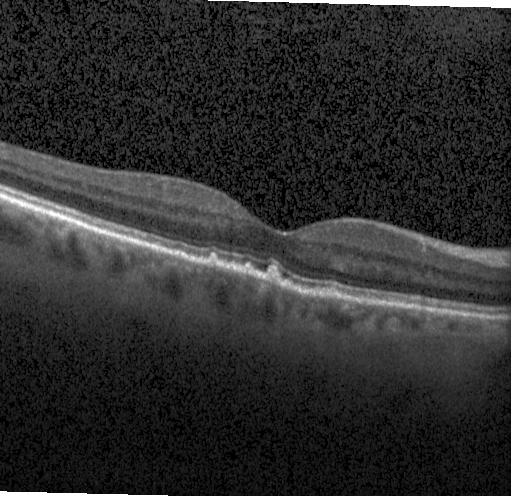
Diagnosis: multiple drusen.